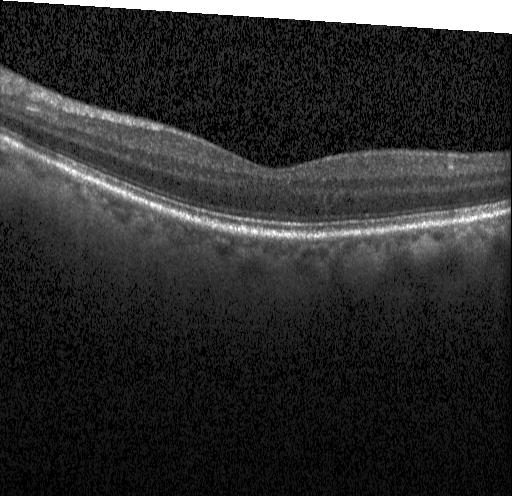

Spectral-domain OCT B-scan: no choroidal neovascularization, diabetic macular edema, or drusen.